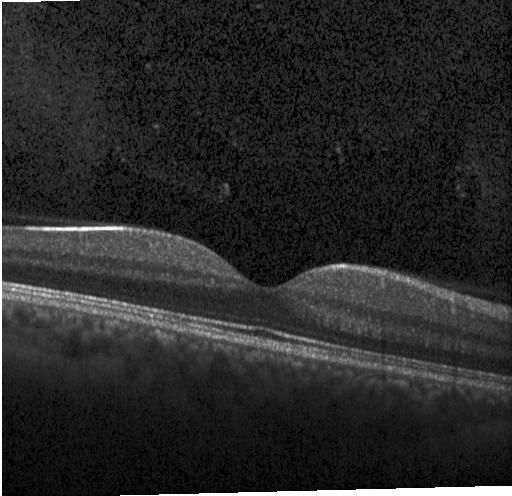 Optical coherence tomography B-scan; SD-OCT
Finding: no evidence of choroidal neovascularization, diabetic macular edema, or drusen.